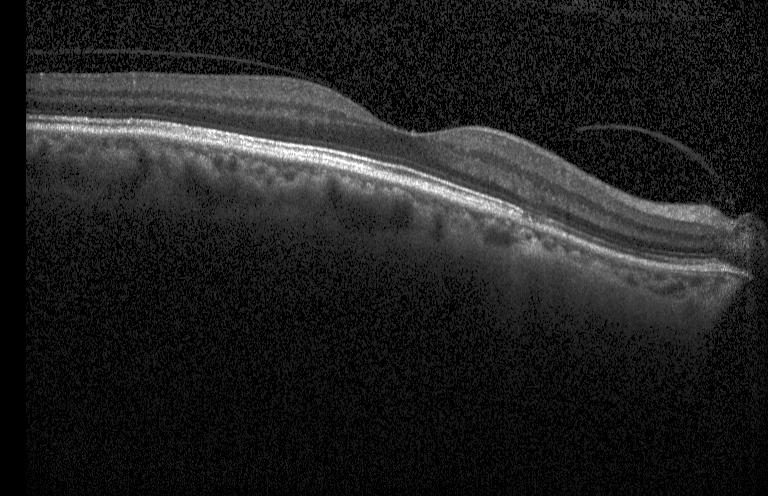
Macular OCT demonstrating no choroidal neovascularization, no diabetic macular edema, and no drusen.